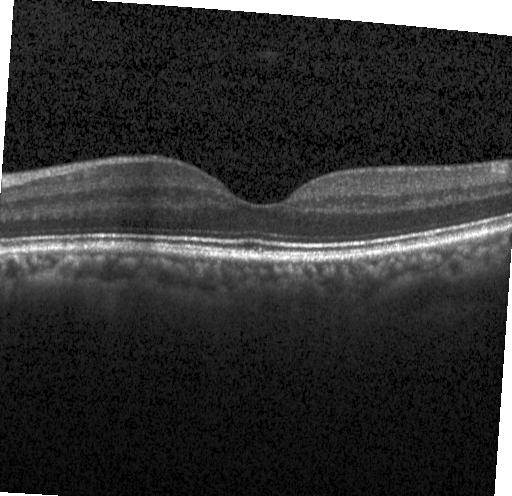 Heidelberg Spectralis. Spectral-domain OCT. Optical coherence tomography B-scan. Fovea-centered — Diagnosis: no CNV, DME, or drusen.